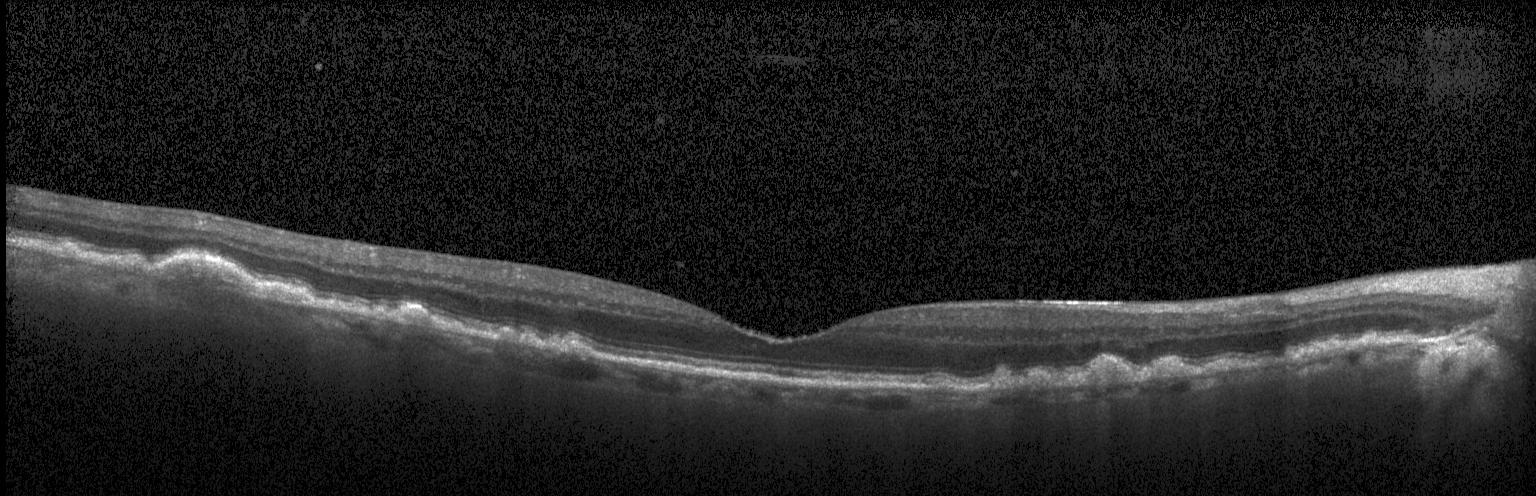
Instrument: Heidelberg Spectralis, optical coherence tomography scan, centered on the fovea.
This B-scan demonstrates sub-RPE drusenoid deposits.